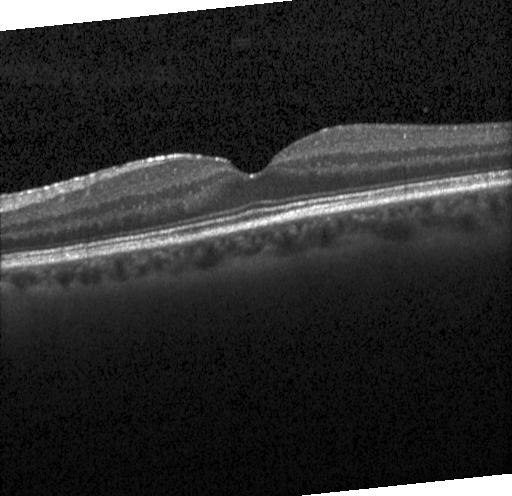
Finding: no CNV, no DME, and no drusen.